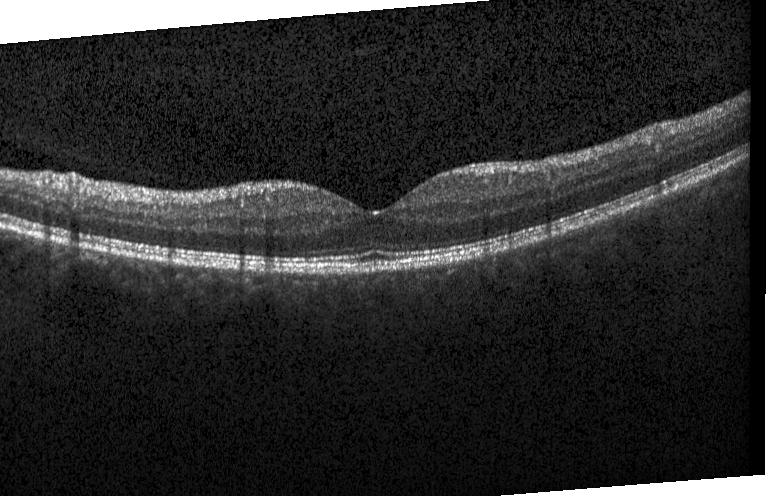

Optical coherence tomography B-scan; acquired on a Heidelberg Spectralis; centered on the fovea.
Finding: no choroidal neovascularization, no diabetic macular edema, and no drusen.